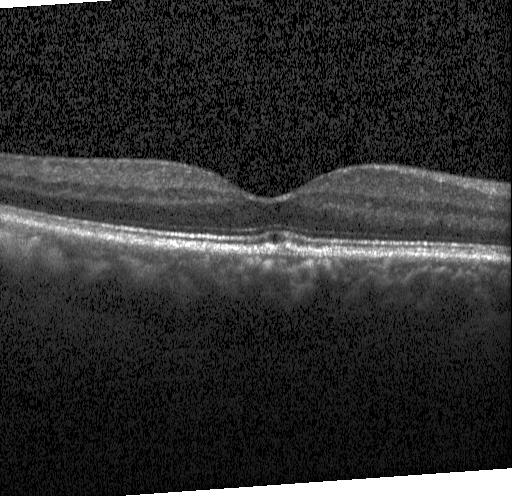
This B-scan demonstrates no choroidal neovascularization, no diabetic macular edema, and no drusen.